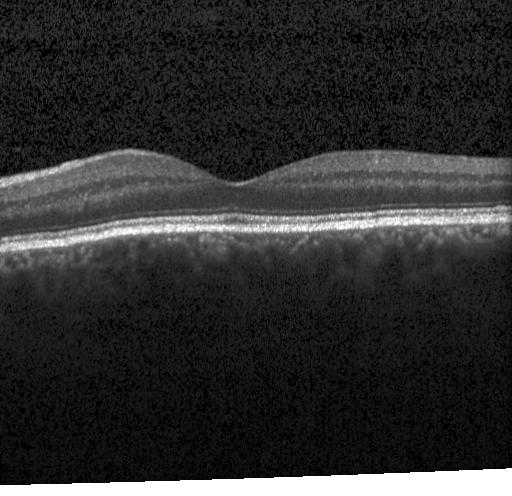
Diagnosis: no choroidal neovascularization, no diabetic macular edema, and no drusen.